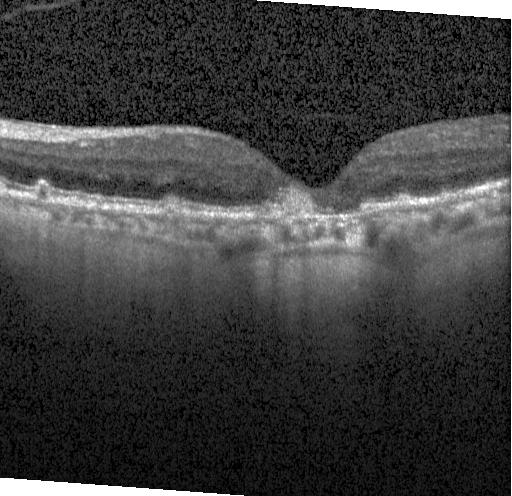

Optical coherence tomography B-scan · spectral-domain OCT.
The scan shows choroidal neovascularization (CNV).